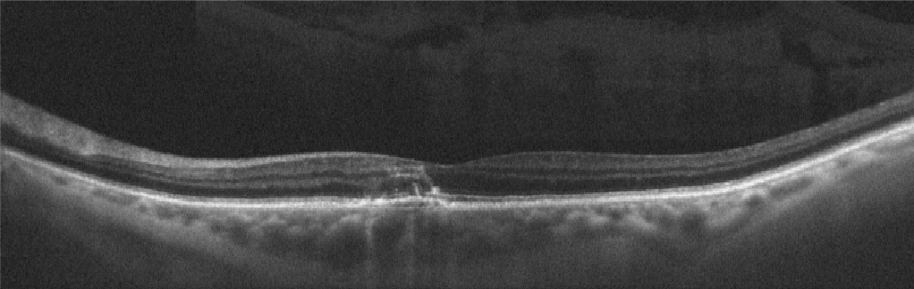
Impression: age-related macular degeneration.